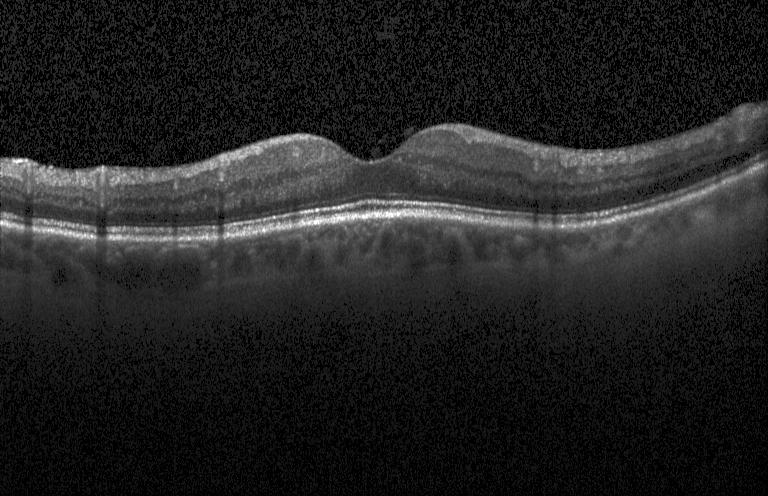
Heidelberg Spectralis OCT system · macular scan · retinal OCT B-scan. Impression: neither CNV, DME, nor drusen.